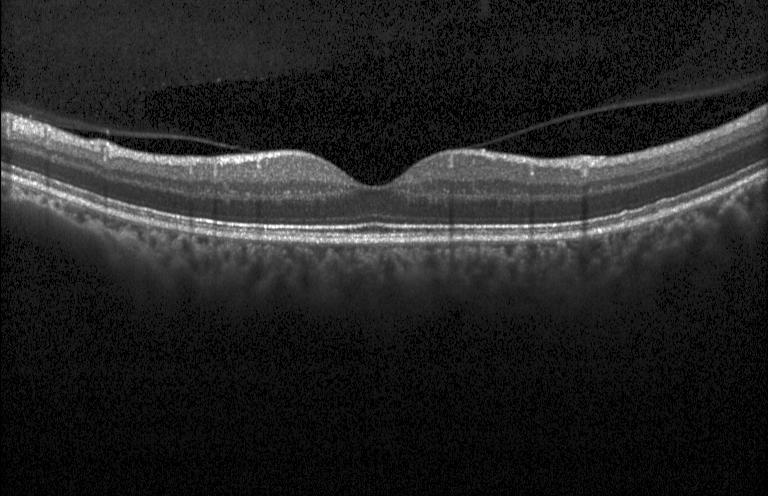

Acquired on a Heidelberg Spectralis · spectral-domain OCT · horizontal scan through the fovea · retinal OCT B-scan
Diagnosis: no evidence of choroidal neovascularization, diabetic macular edema, or drusen.